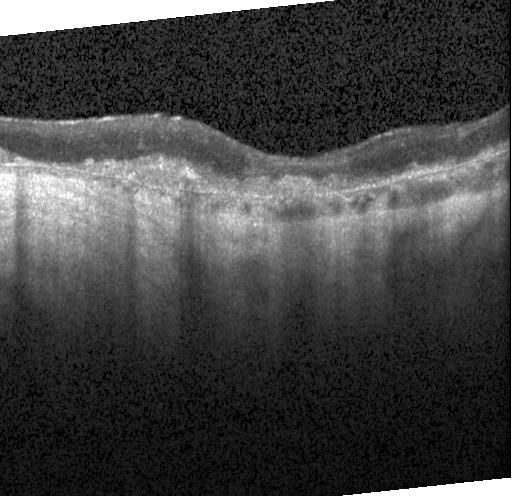 Finding: CNV.